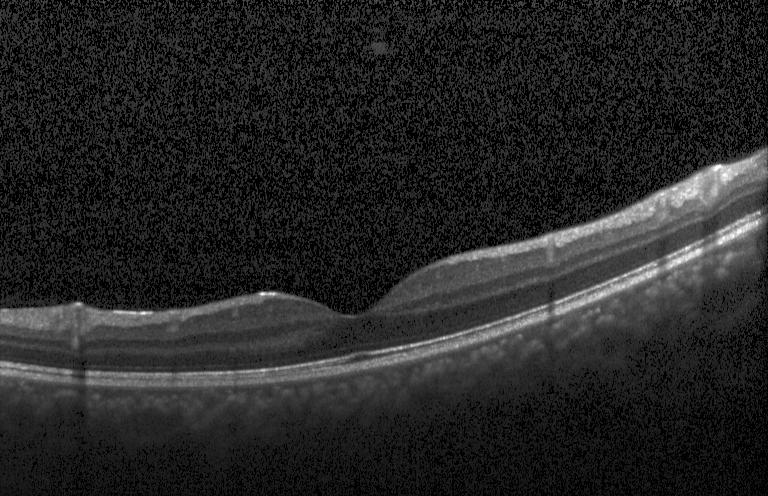
Macular OCT demonstrating no choroidal neovascularization, diabetic macular edema, or drusen.